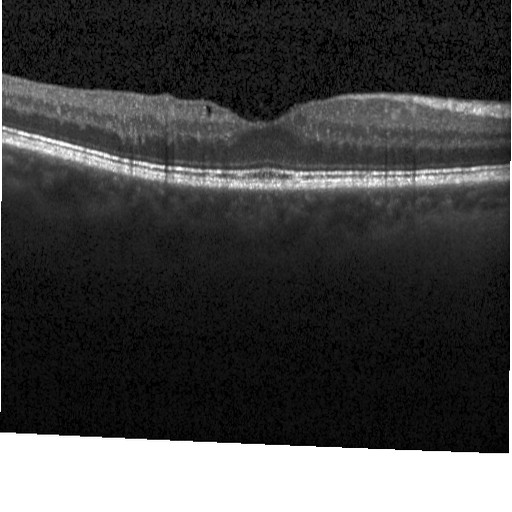
Optical coherence tomography B-scan. Spectral-domain optical coherence tomography. Centered on the fovea. Acquired on a Heidelberg Spectralis. OCT finding: DME.